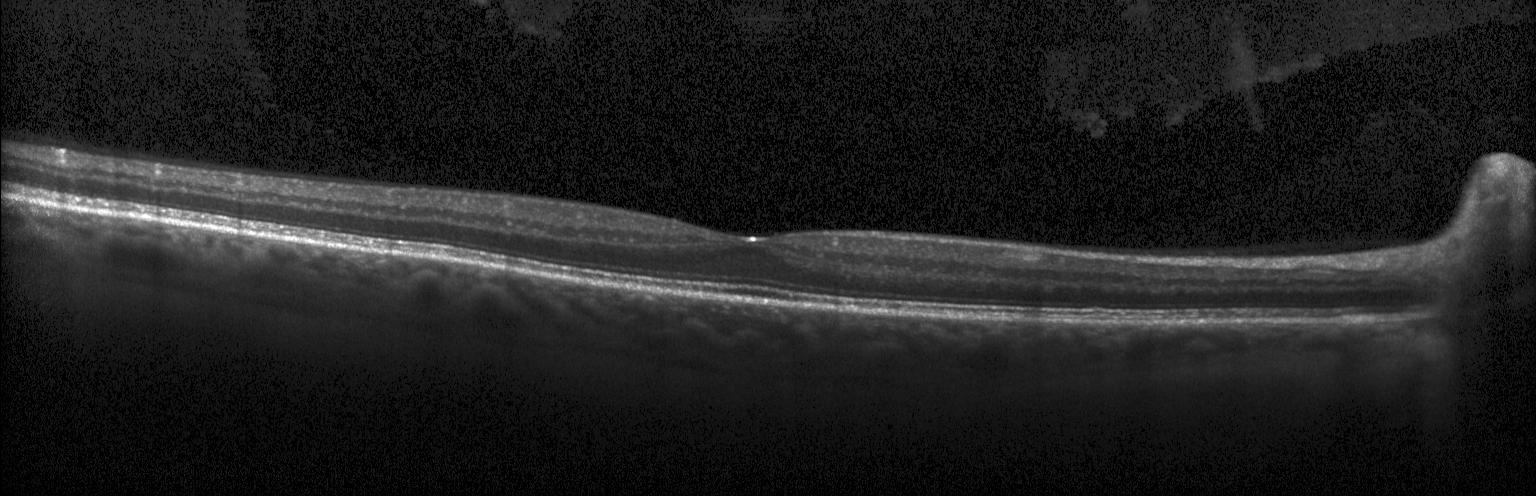
Retinal OCT B-scan — Dx: no choroidal neovascularization, diabetic macular edema, or drusen.